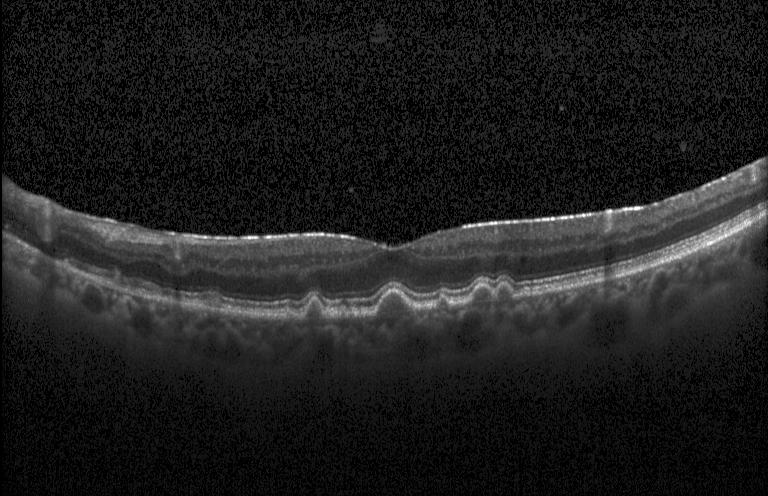
Spectral-domain optical coherence tomography; OCT B-scan.
Diagnosis: multiple drusen.